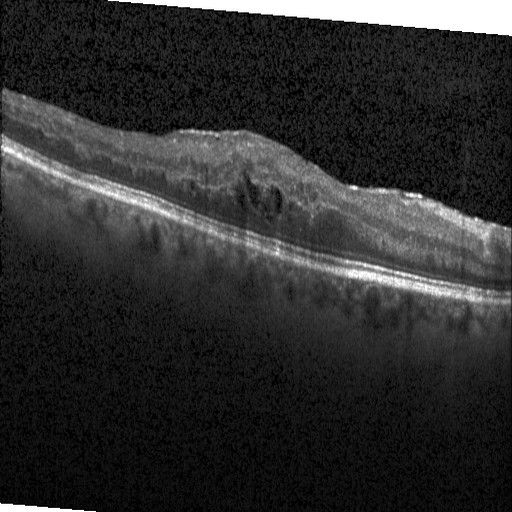

Optical coherence tomography B-scan; SD-OCT. Assessment: diabetic macular edema (DME).